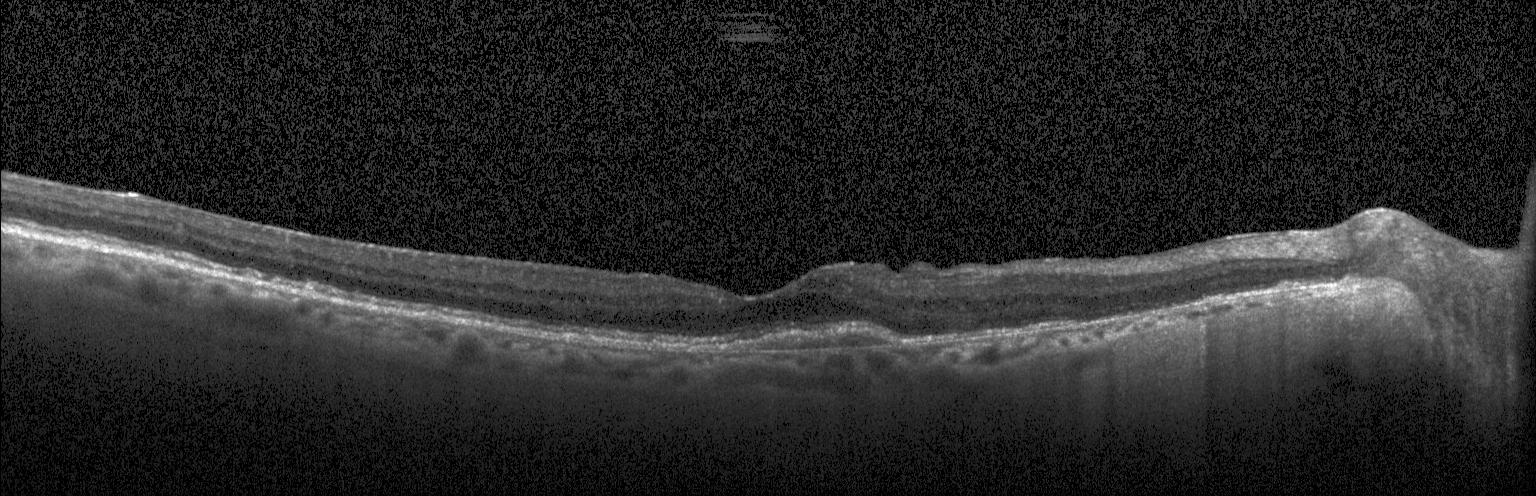
Instrument: Heidelberg Spectralis. SD-OCT. OCT line scan — OCT finding: choroidal neovascularization.